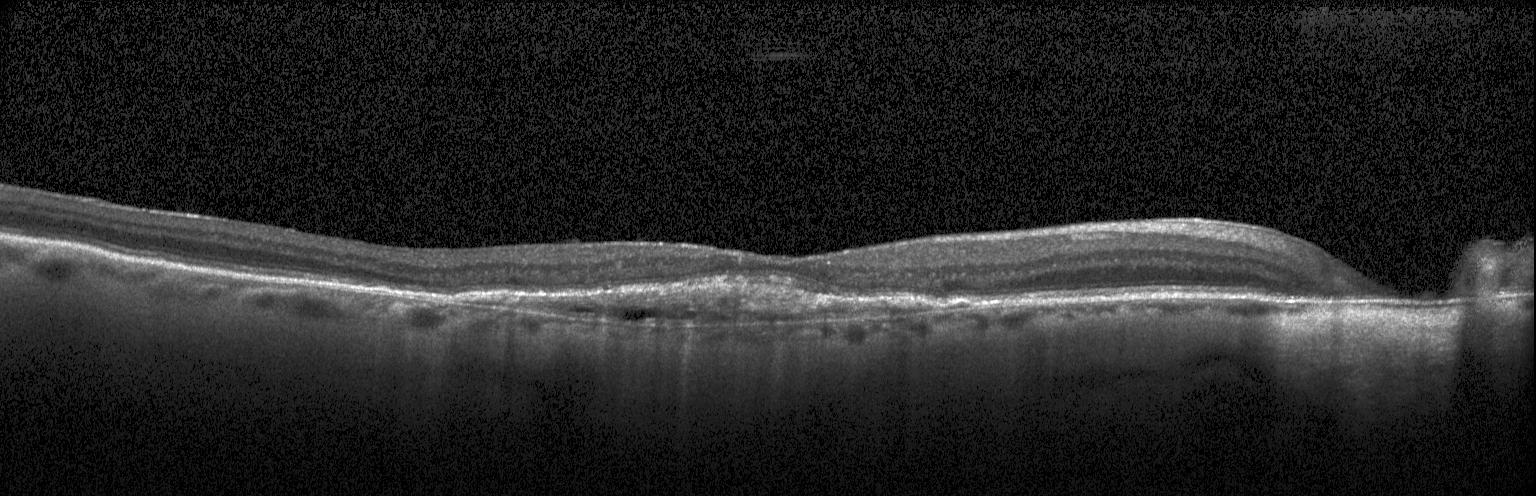
SD-OCT. Optical coherence tomography scan. Through the macula.
A choroidal neovascular membrane.